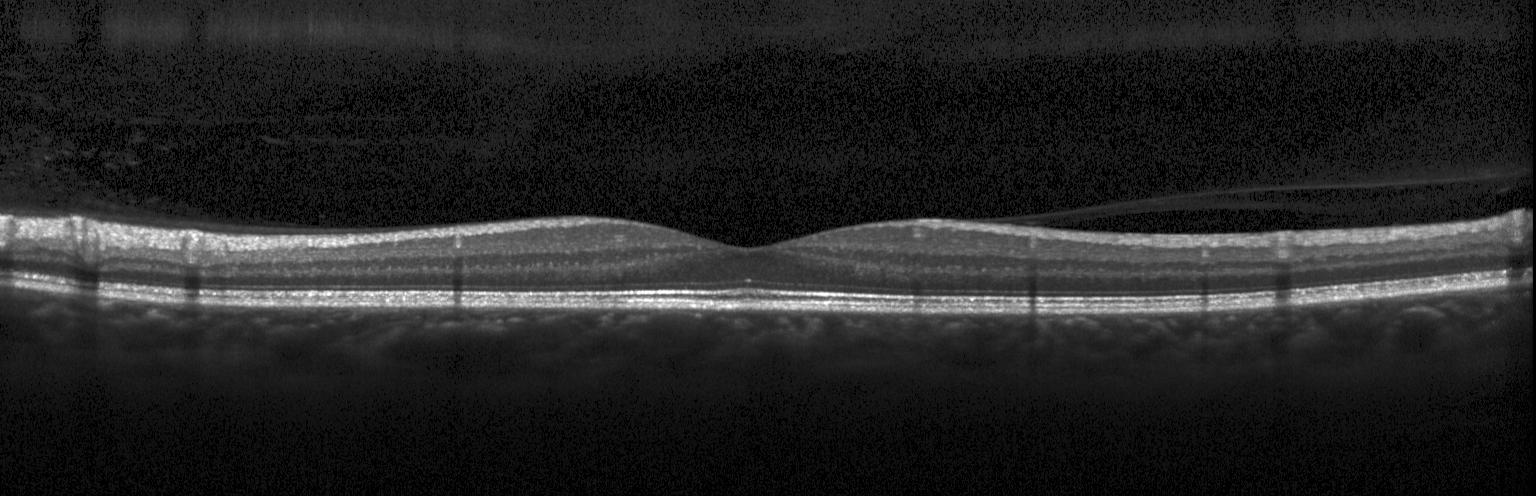

Optical coherence tomography scan, SD-OCT, Heidelberg Spectralis OCT system. No CNV, DME, or drusen.